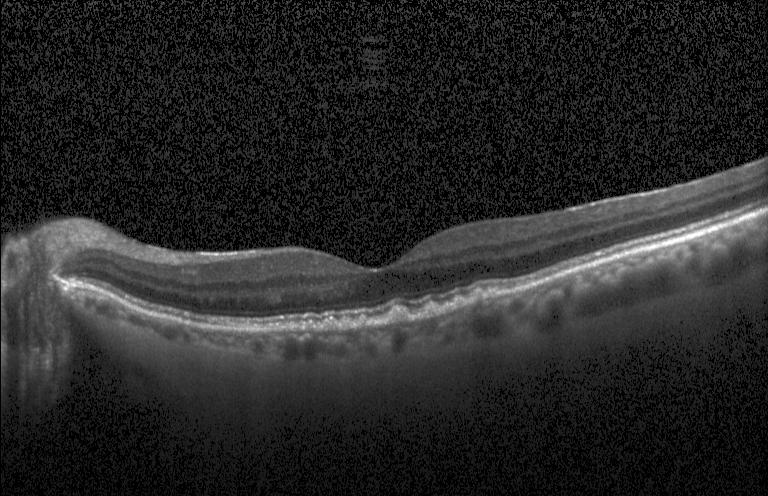 OCT B-scan · fovea-centered · Heidelberg Spectralis.
Diagnosis: drusen.